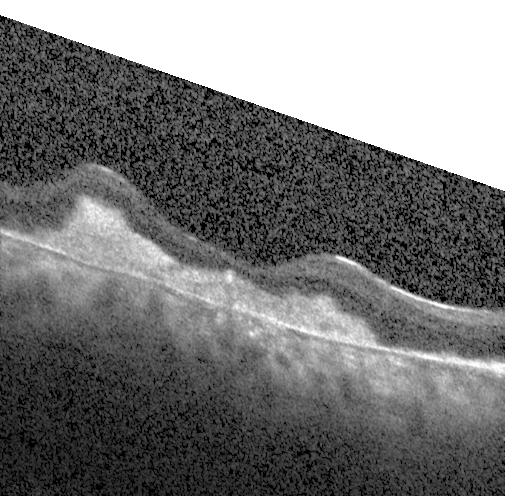

Dx: CNV.